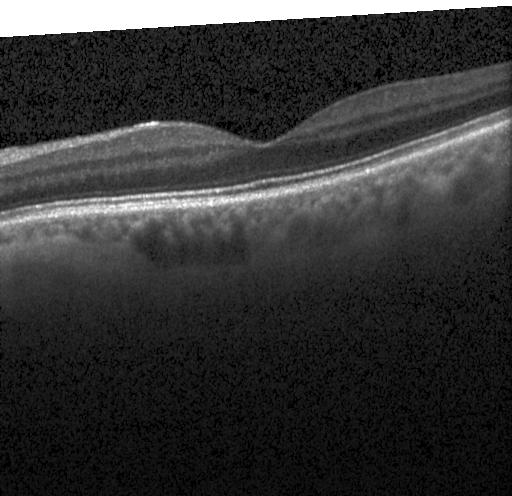

Dx: no evidence of choroidal neovascularization, diabetic macular edema, or drusen.